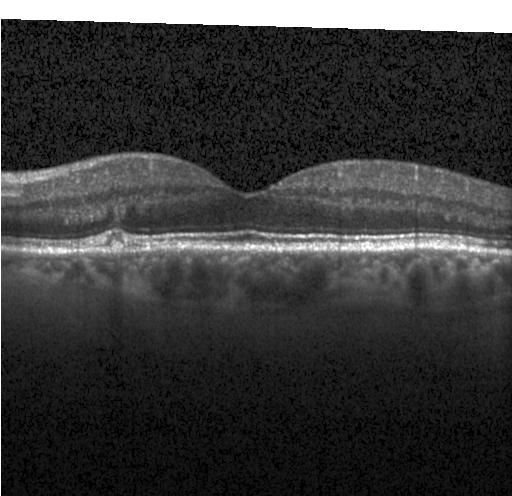
Macular OCT: drusen.